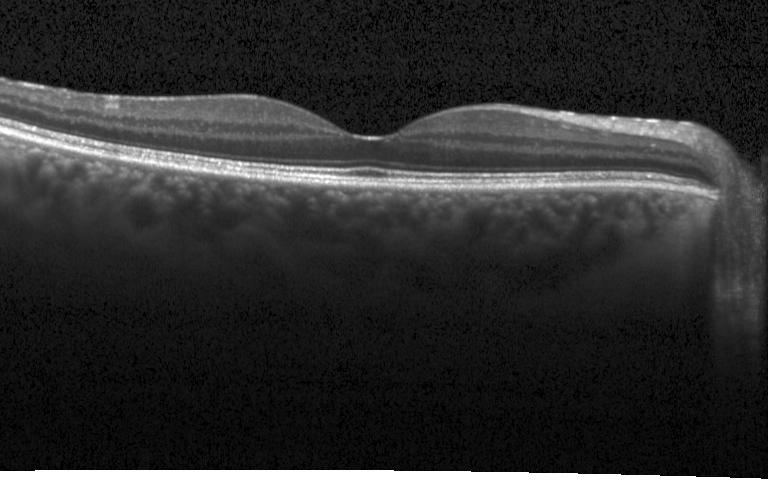
Finding: neither choroidal neovascularization, diabetic macular edema, nor drusen.